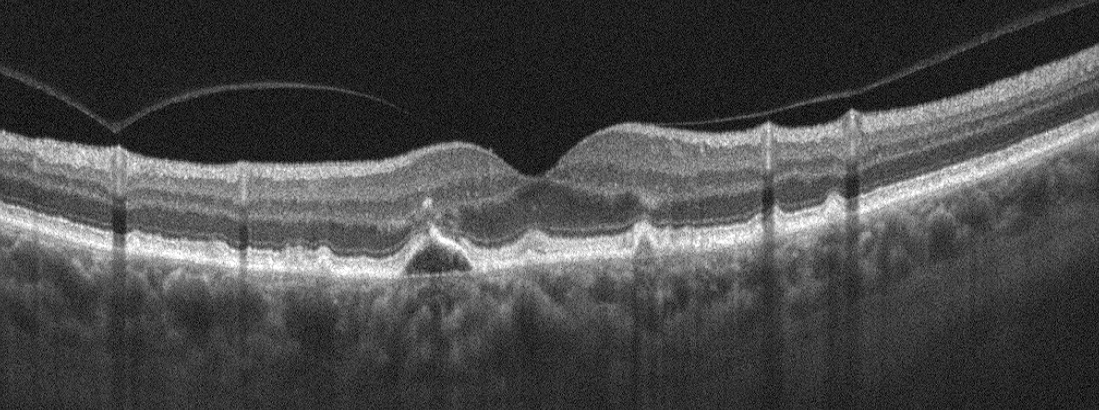 Optical coherence tomography B-scan. Instrument: Optovue Avanti RTVue XR.
Age-related macular degeneration (AMD).